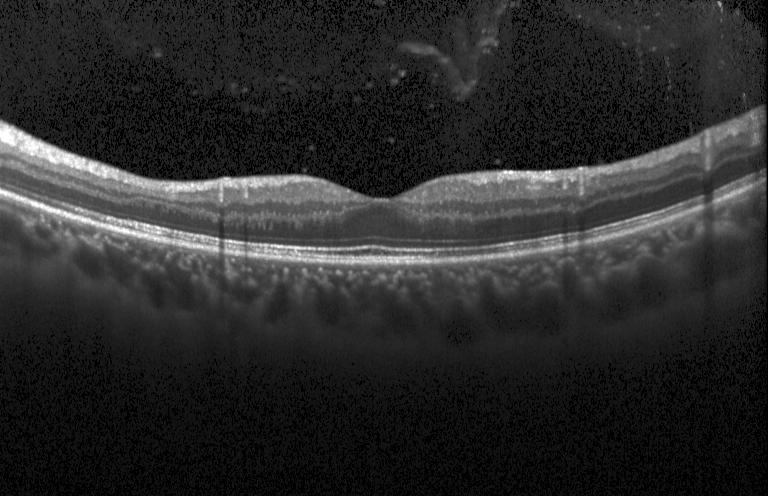 Macular OCT demonstrating neither choroidal neovascularization, diabetic macular edema, nor drusen.